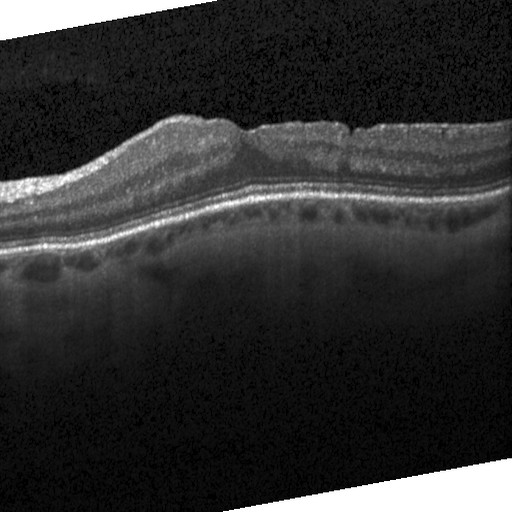

Retinal OCT B-scan. This B-scan demonstrates diabetic macular edema.